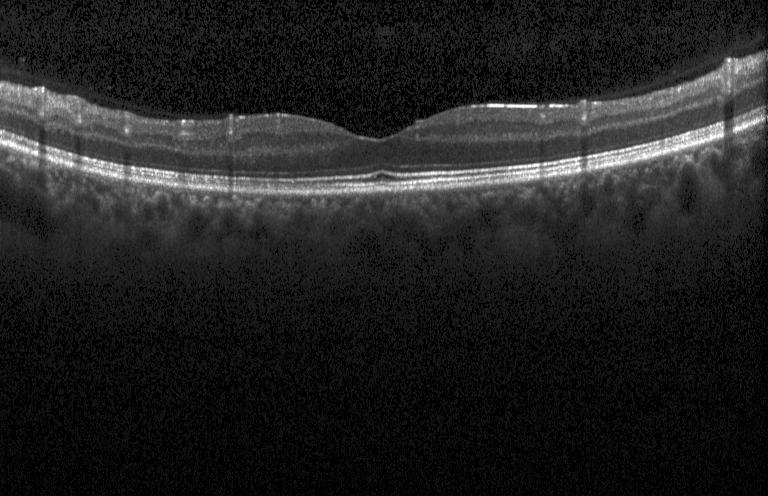

OCT finding: no evidence of CNV, DME, or drusen.